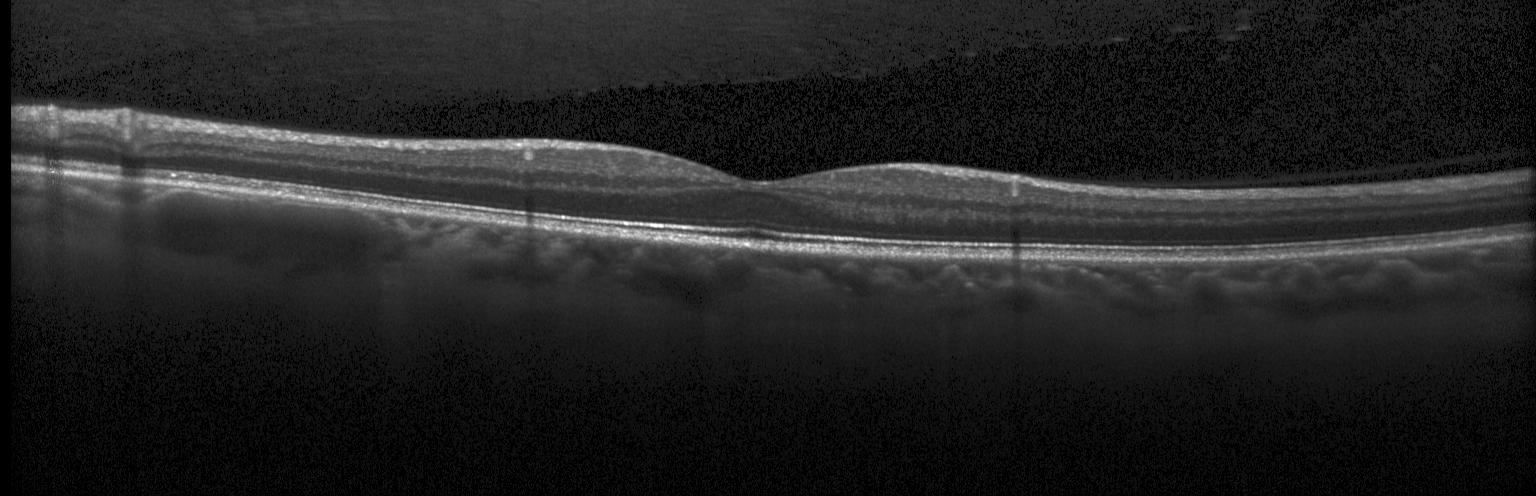 Instrument: Heidelberg Spectralis · optical coherence tomography scan. The scan shows no evidence of choroidal neovascularization, diabetic macular edema, or drusen.